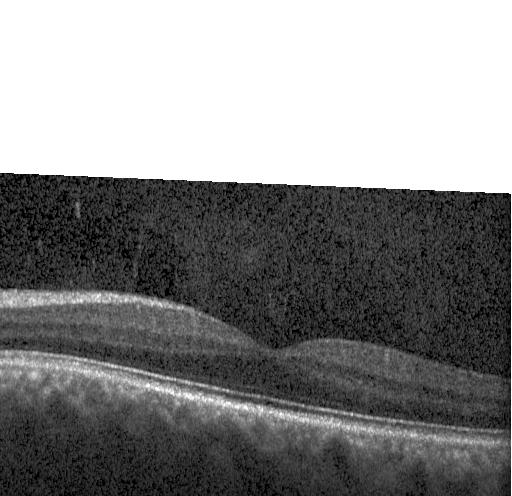 OCT B-scan. Centered on the fovea.
Assessment: no CNV, no DME, and no drusen.